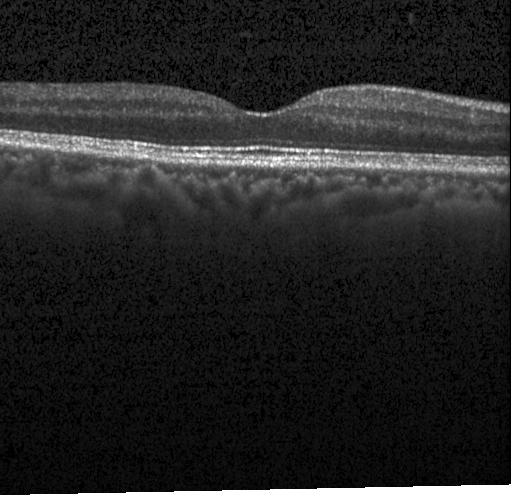

Retinal OCT B-scan · instrument: Heidelberg Spectralis
The scan shows neither choroidal neovascularization, diabetic macular edema, nor drusen.